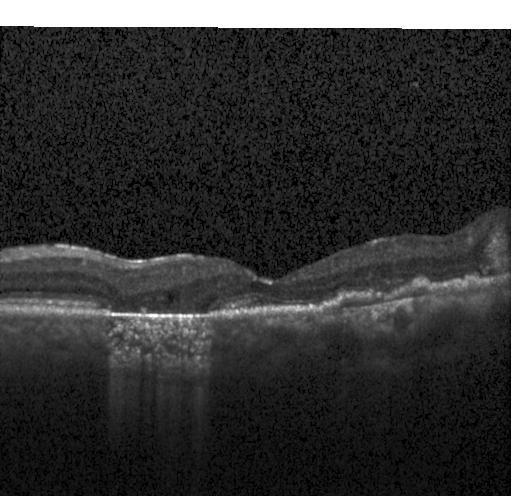 Spectral-domain optical coherence tomography · acquired on a Heidelberg Spectralis · retinal OCT B-scan
Macular OCT: a choroidal neovascular membrane.